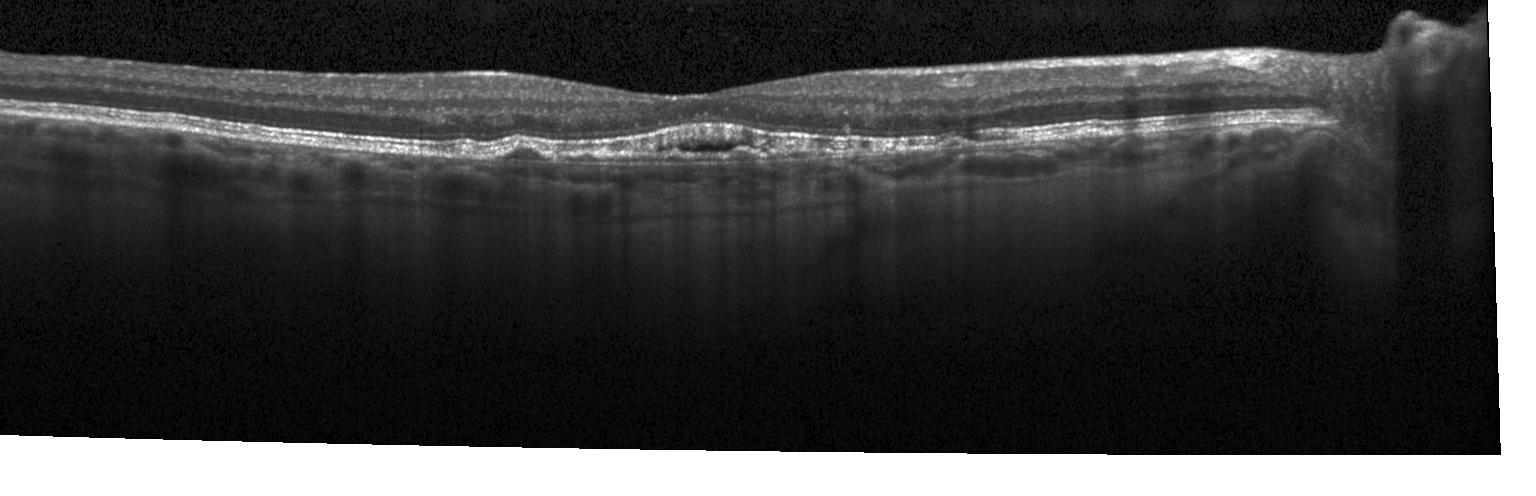

OCT scan showing choroidal neovascularization.